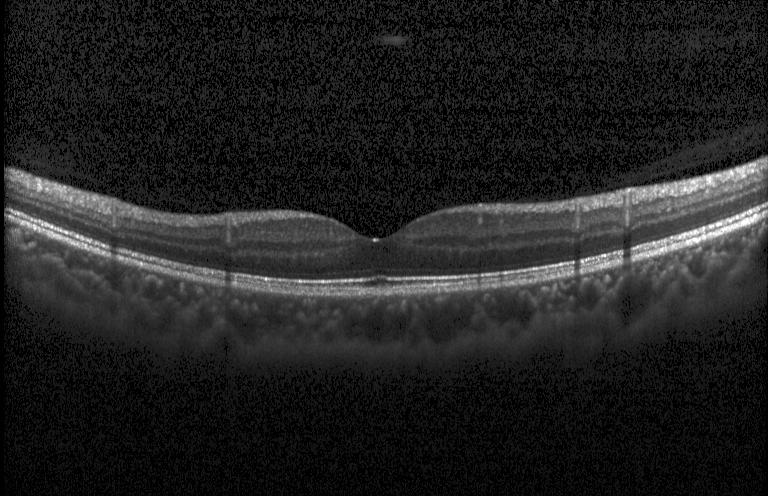

Retinal OCT B-scan. SD-OCT. Centered on the fovea.
OCT finding: neither choroidal neovascularization, diabetic macular edema, nor drusen.